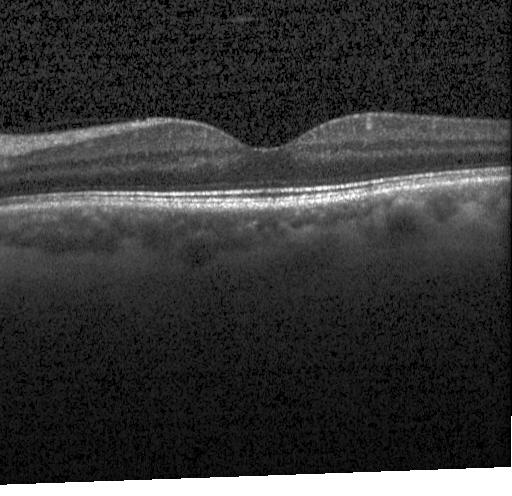
Fovea-centered. SD-OCT. Retinal OCT cross-section
Diagnosis: neither CNV, DME, nor drusen.